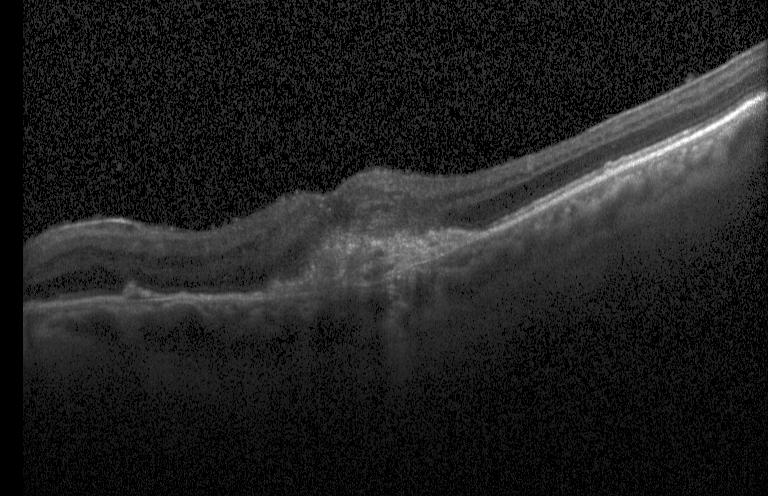

Through the macula; retinal OCT B-scan — Finding: a choroidal neovascular membrane.